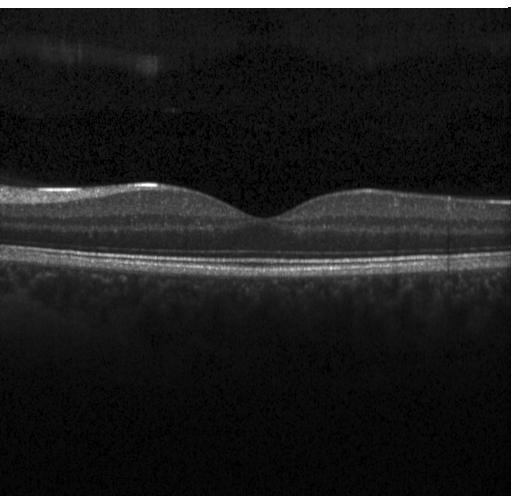
Optical coherence tomography B-scan; SD-OCT; acquired on a Heidelberg Spectralis; horizontal scan through the fovea — Diagnosis: neither choroidal neovascularization, diabetic macular edema, nor drusen.